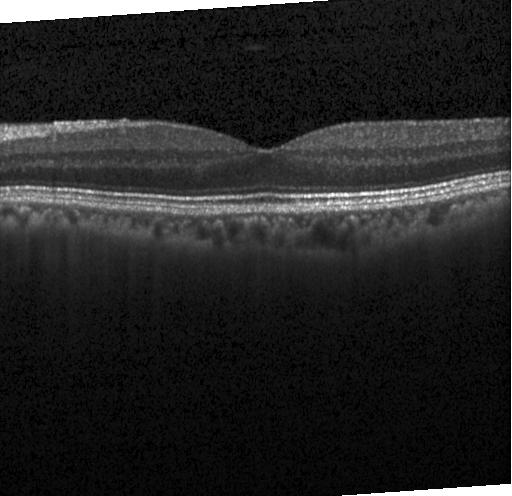 This B-scan demonstrates no choroidal neovascularization, diabetic macular edema, or drusen.